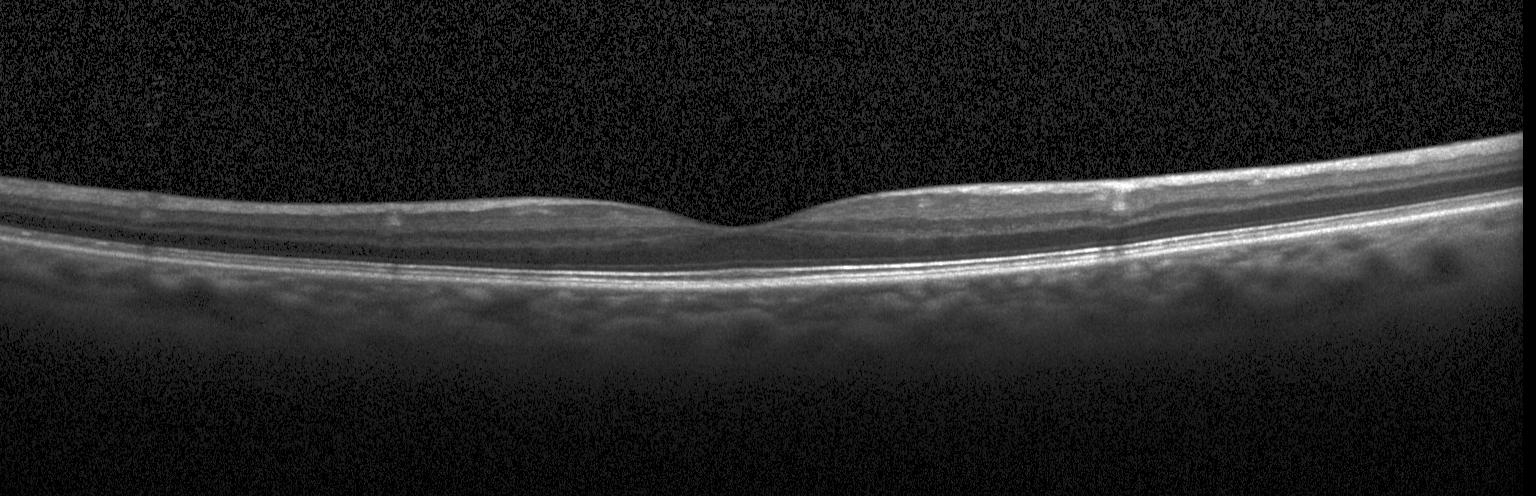 Optical coherence tomography scan · Heidelberg Spectralis · spectral-domain optical coherence tomography · horizontal scan through the fovea
Impression: no choroidal neovascularization, no diabetic macular edema, and no drusen.